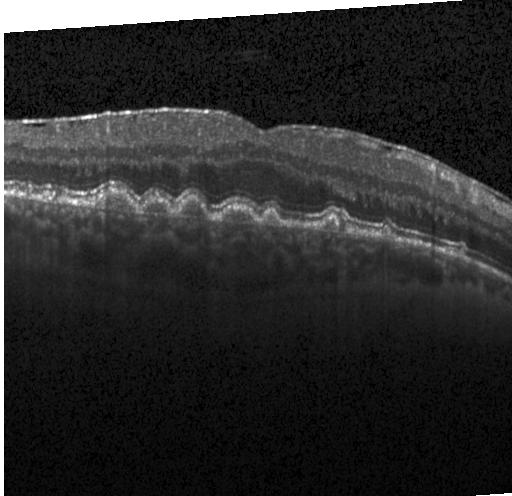

Retinal OCT B-scan · fovea-centered. Macular OCT: drusen.